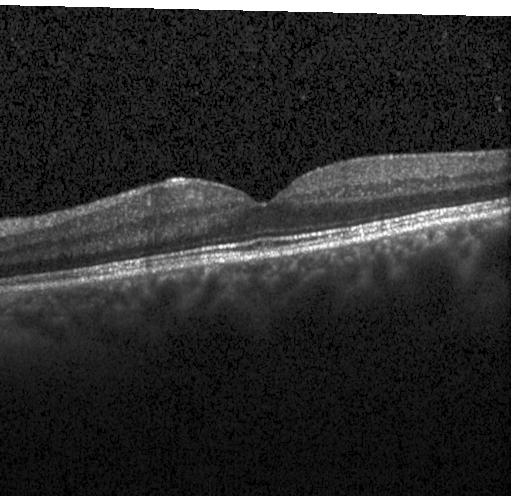
Optical coherence tomography B-scan, fovea-centered, spectral-domain optical coherence tomography
Impression: no CNV, DME, or drusen.